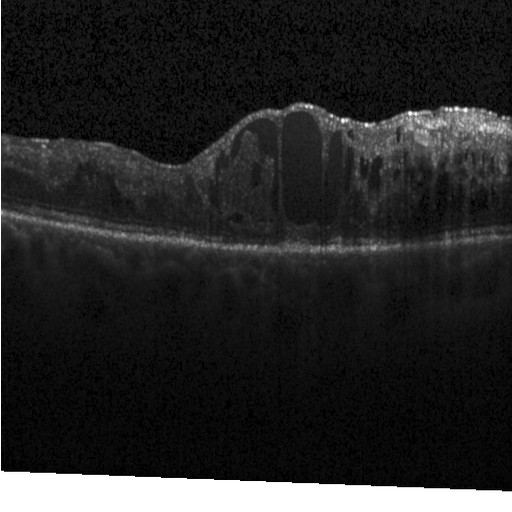
Centered on the fovea. Retinal OCT cross-section. Heidelberg Spectralis OCT system. SD-OCT.
This B-scan demonstrates DME.